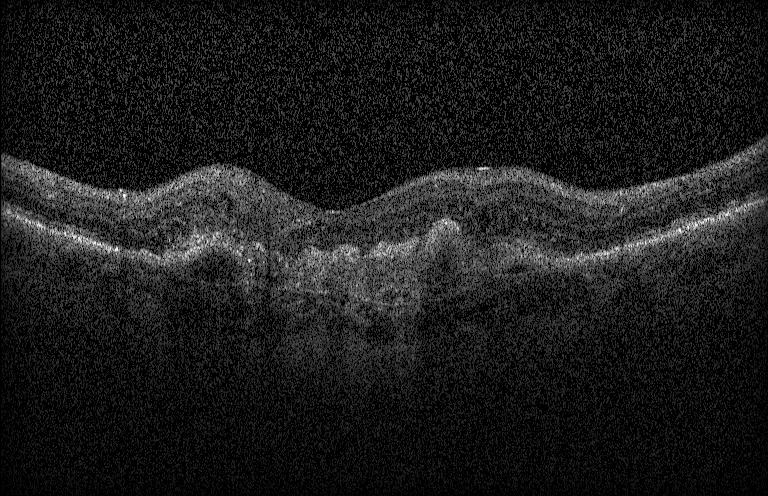 Retinal OCT cross-section — Finding: choroidal neovascularization (CNV).